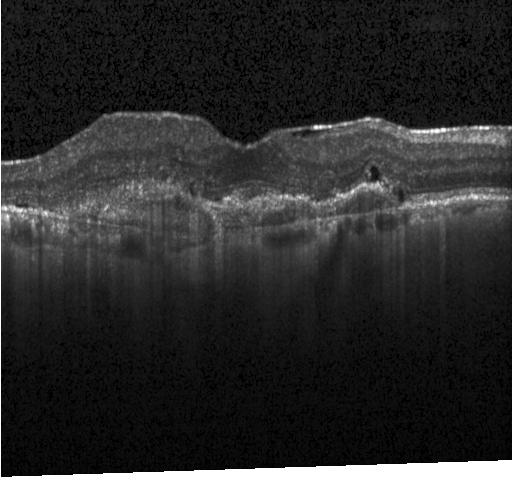 Impression: CNV.